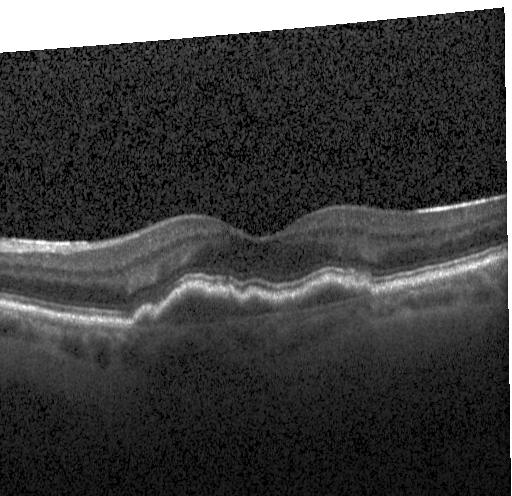
OCT line scan · fovea-centered · Heidelberg Spectralis OCT system. Finding: CNV.